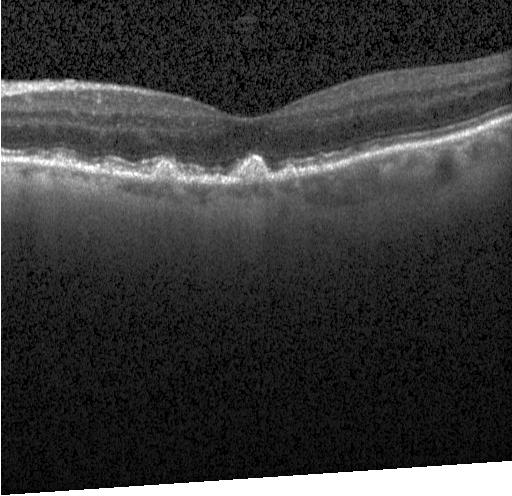
Centered on the fovea; OCT B-scan; Heidelberg Spectralis OCT system; SD-OCT. Assessment: sub-RPE drusenoid deposits.